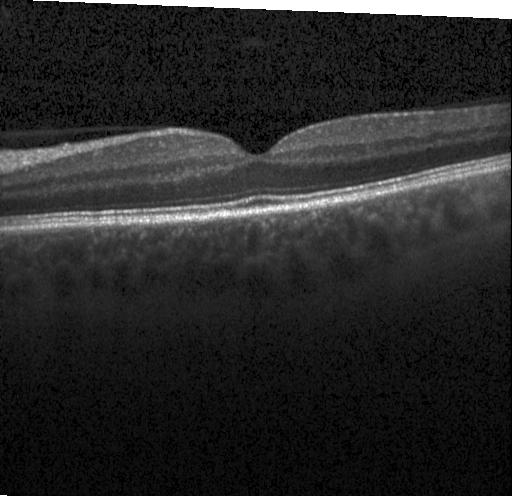
Retinal OCT B-scan · spectral-domain OCT · fovea-centered. Diagnosis: no choroidal neovascularization, no diabetic macular edema, and no drusen.